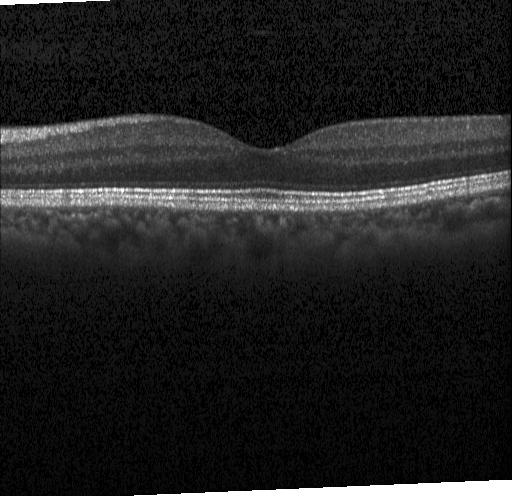
Instrument: Heidelberg Spectralis · spectral-domain OCT · macular scan · retinal OCT B-scan — Diagnosis: no CNV, DME, or drusen.